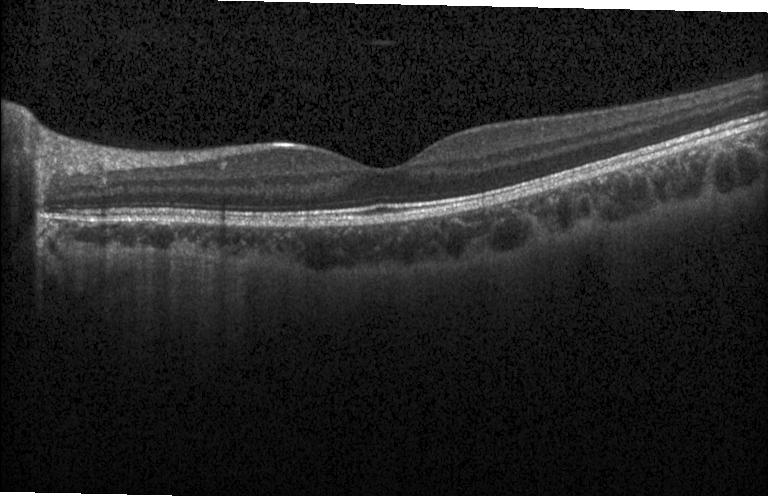

Macular scan; retinal OCT B-scan; spectral-domain optical coherence tomography
The scan shows no choroidal neovascularization, no diabetic macular edema, and no drusen.